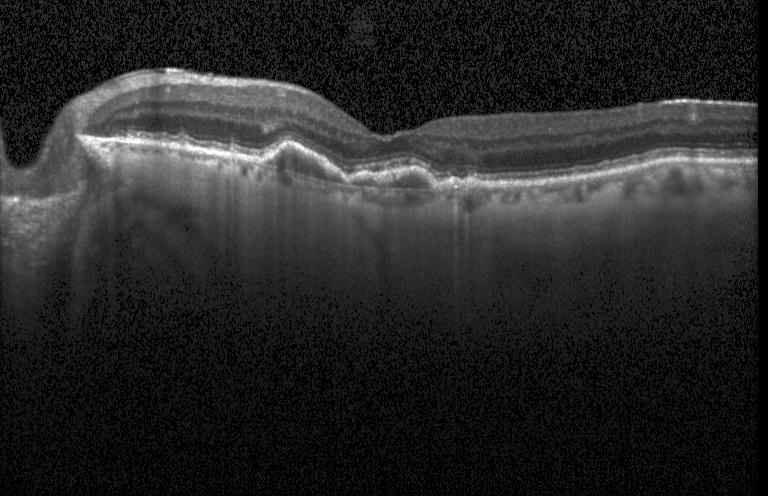
Diagnosis: a choroidal neovascular membrane.